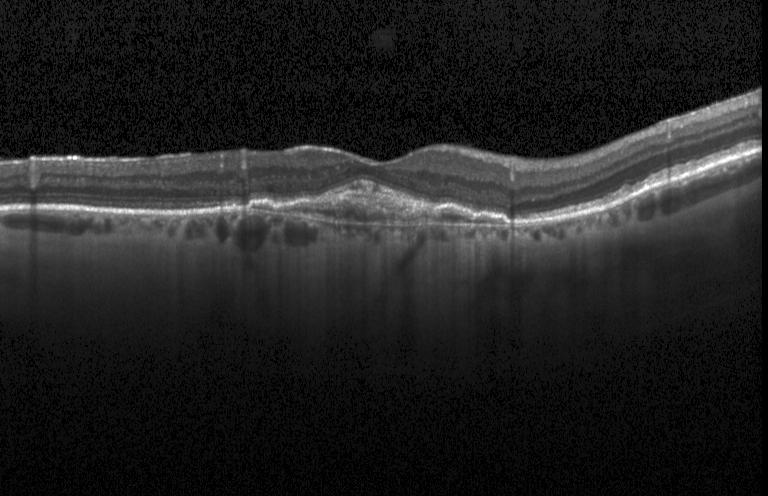 Heidelberg Spectralis OCT system, optical coherence tomography B-scan.
Dx: a choroidal neovascular membrane.